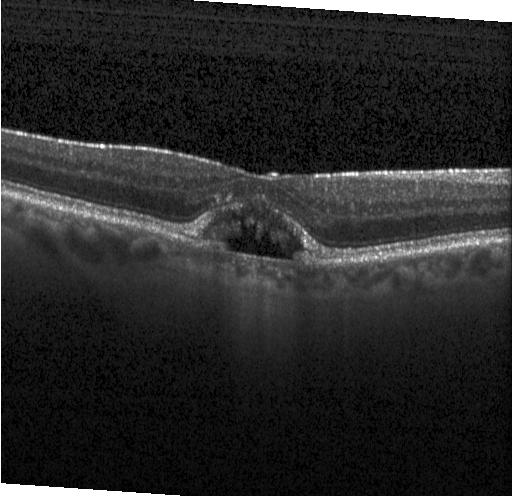

The scan shows a choroidal neovascular membrane.